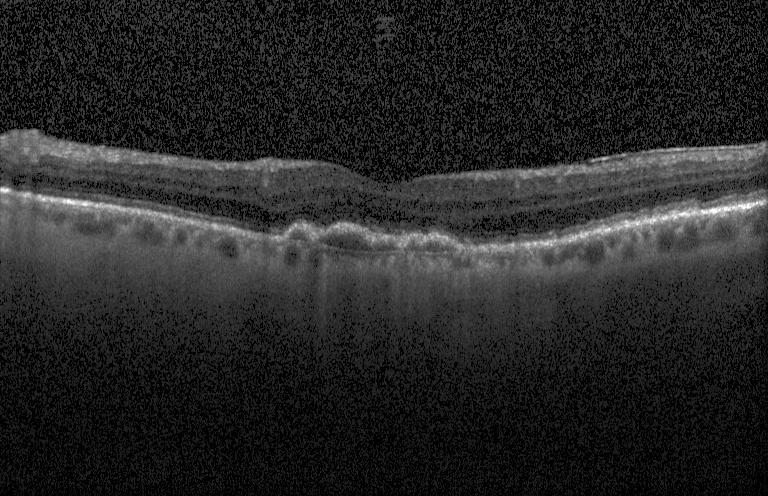 Retinal OCT B-scan
Macular OCT: CNV.